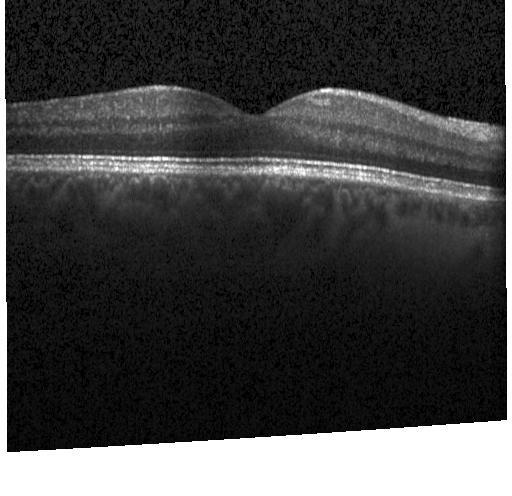

Spectral-domain optical coherence tomography; fovea-centered; OCT B-scan; acquired on a Heidelberg Spectralis — Finding: no choroidal neovascularization, no diabetic macular edema, and no drusen.